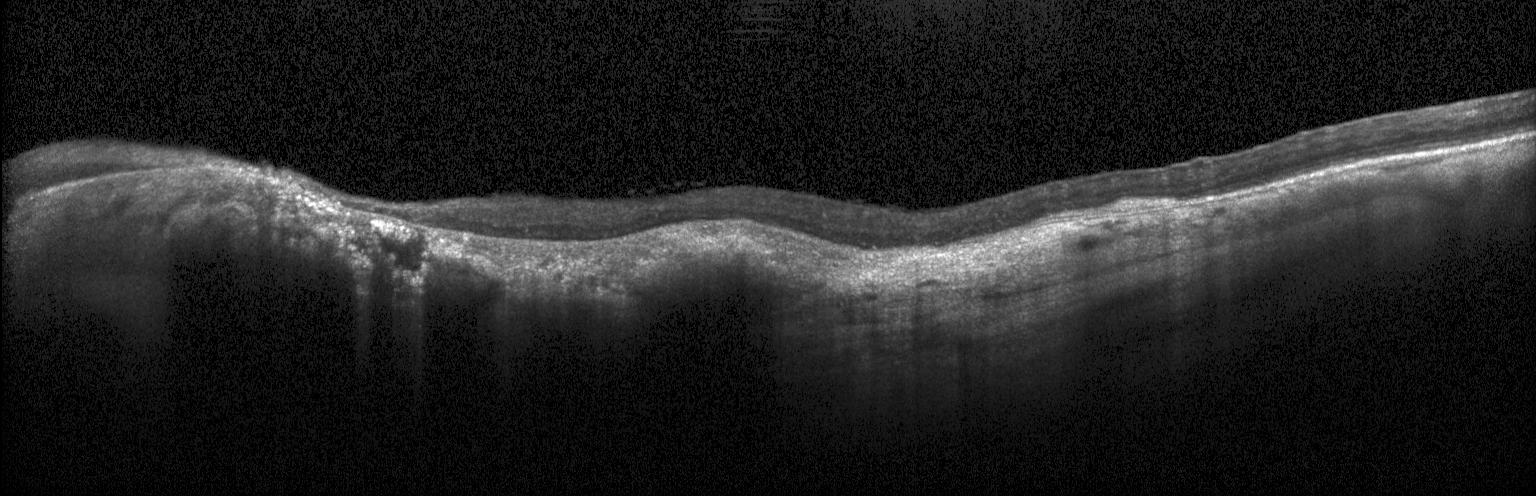

Horizontal scan through the fovea · SD-OCT · optical coherence tomography B-scan · Heidelberg Spectralis OCT system. The scan shows choroidal neovascularization (CNV).